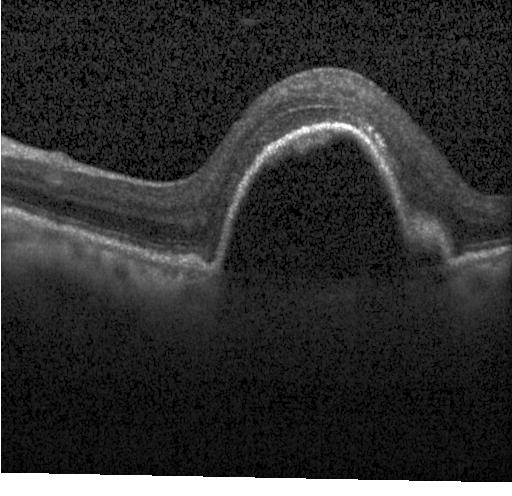
Spectral-domain OCT B-scan: choroidal neovascularization.